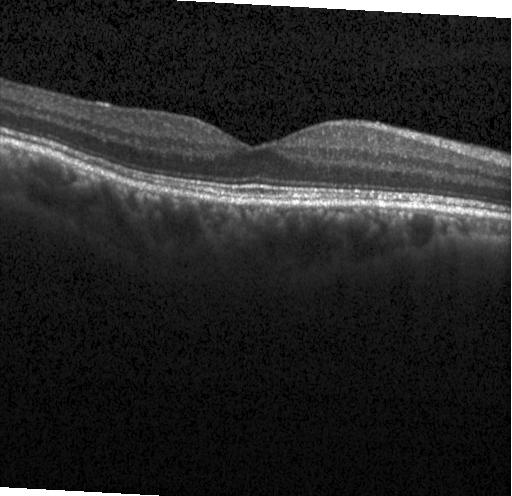 Dx: no evidence of choroidal neovascularization, diabetic macular edema, or drusen.